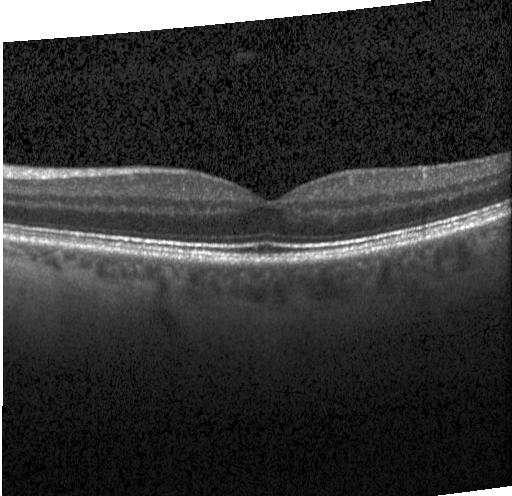

Macular OCT: no CNV, no DME, and no drusen.